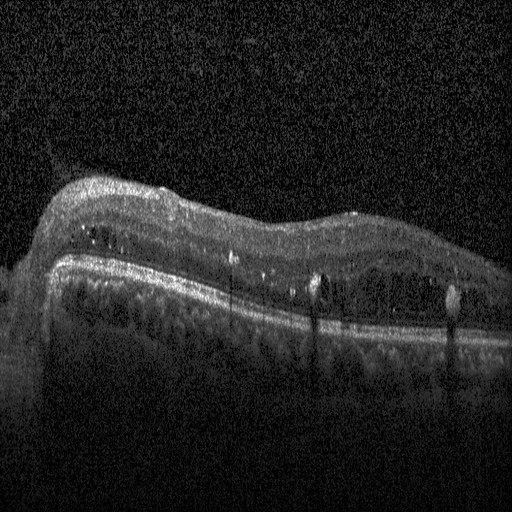
Spectral-domain OCT. Through the macula. Retinal OCT cross-section. Acquired on a Heidelberg Spectralis.
The scan shows diabetic macular edema.